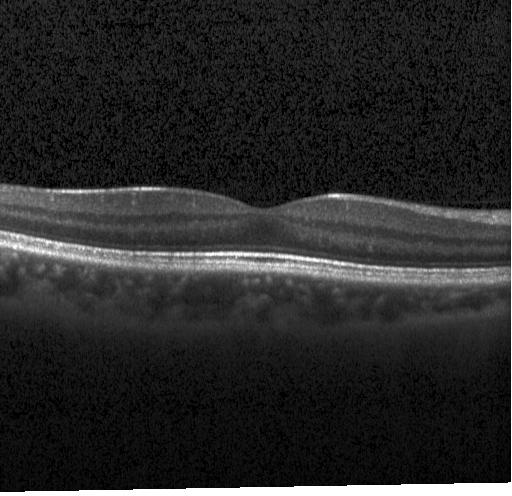

Fovea-centered · SD-OCT · optical coherence tomography scan — The scan shows no evidence of CNV, DME, or drusen.